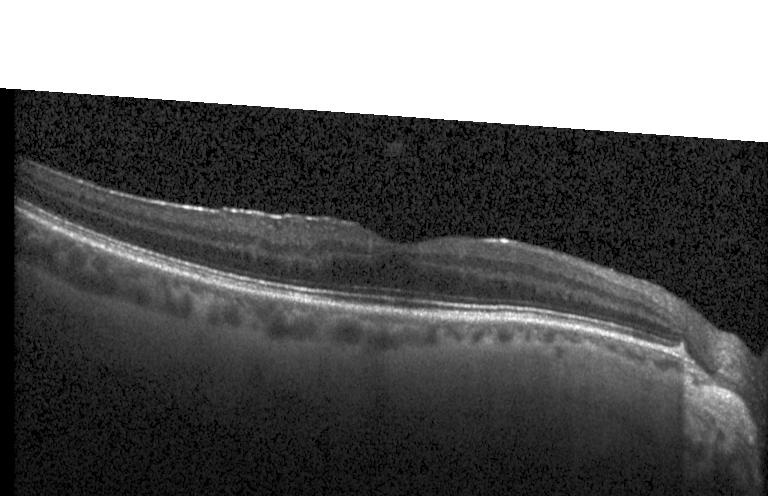

Through the macula; OCT B-scan.
Assessment: no choroidal neovascularization, no diabetic macular edema, and no drusen.